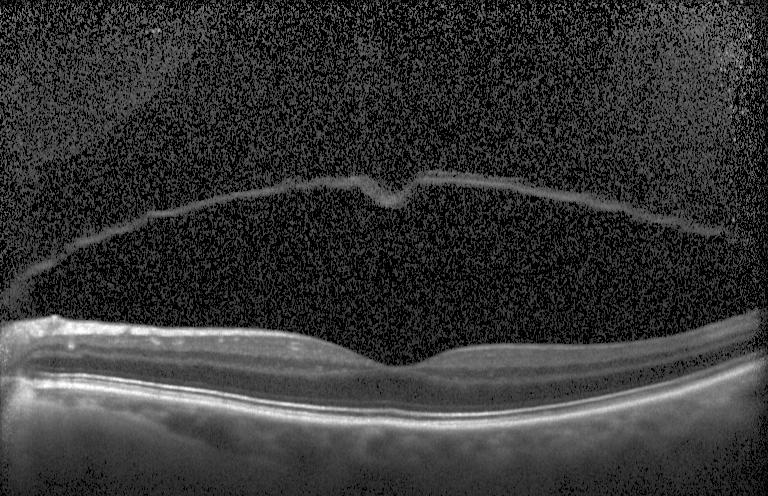

Through the macula; spectral-domain OCT; retinal OCT cross-section
Finding: no CNV, DME, or drusen.